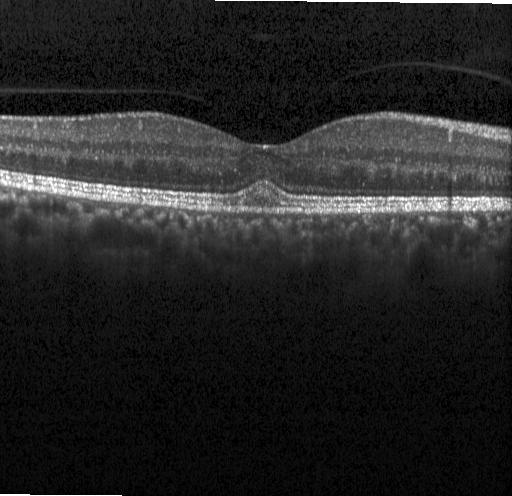

Acquired on a Heidelberg Spectralis · optical coherence tomography scan · fovea-centered
Impression: CNV.